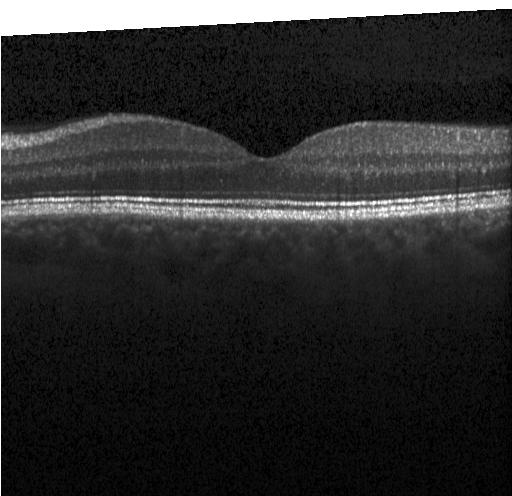 Retinal OCT cross-section showing neither choroidal neovascularization, diabetic macular edema, nor drusen.